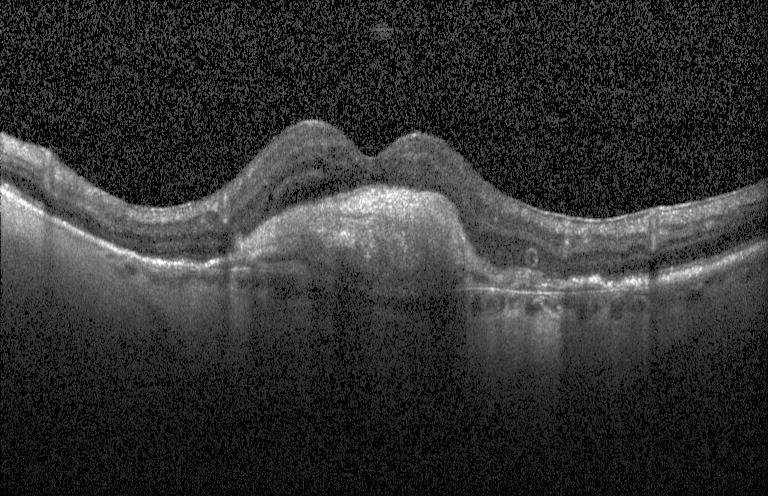 Instrument: Heidelberg Spectralis; SD-OCT; optical coherence tomography B-scan; fovea-centered.
OCT finding: CNV.